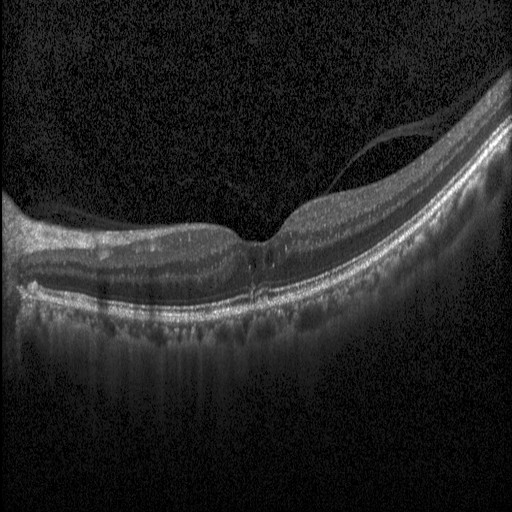 Through the macula · OCT B-scan · Heidelberg Spectralis OCT system. Assessment: diabetic macular edema (DME).